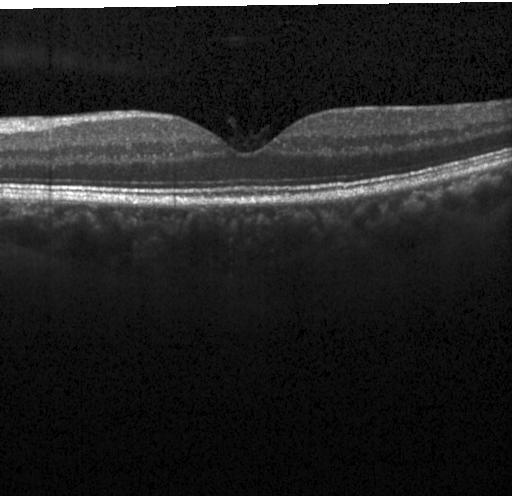 OCT line scan · Heidelberg Spectralis OCT system.
Diagnosis: no evidence of choroidal neovascularization, diabetic macular edema, or drusen.